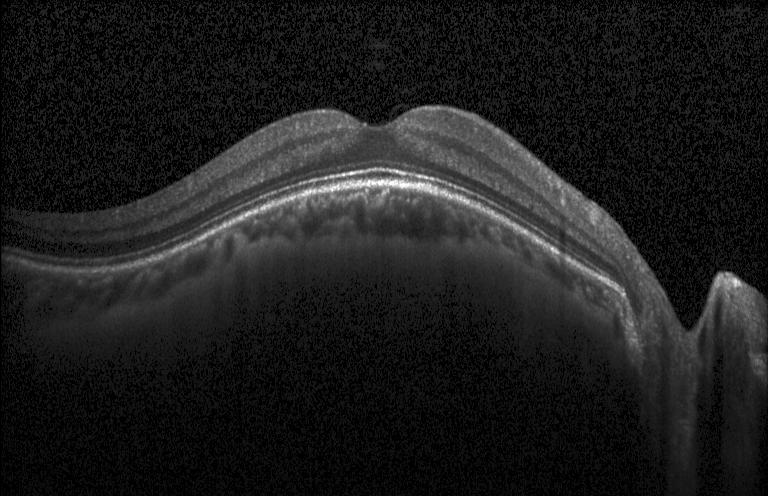 Spectral-domain optical coherence tomography · retinal OCT cross-section · acquired on a Heidelberg Spectralis — No CNV, no DME, and no drusen.